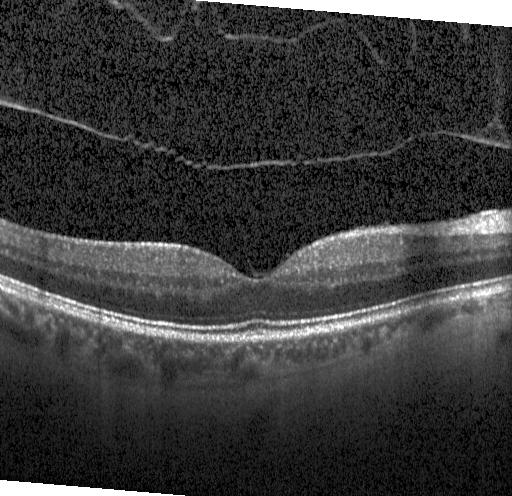
Acquired on a Heidelberg Spectralis; spectral-domain OCT; optical coherence tomography B-scan.
OCT finding: no evidence of choroidal neovascularization, diabetic macular edema, or drusen.